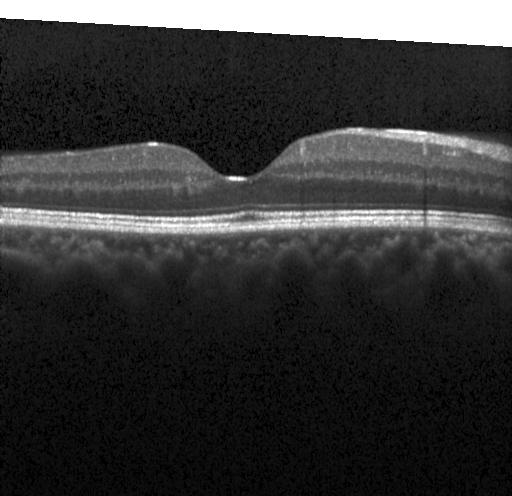

Macular OCT: no evidence of CNV, DME, or drusen.